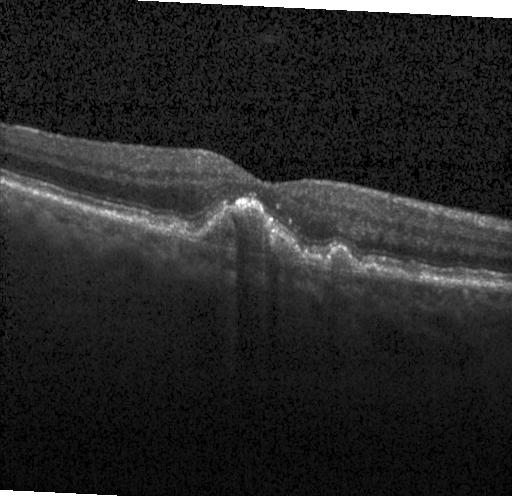 Optical coherence tomography B-scan. Heidelberg Spectralis — Impression: a choroidal neovascular membrane.